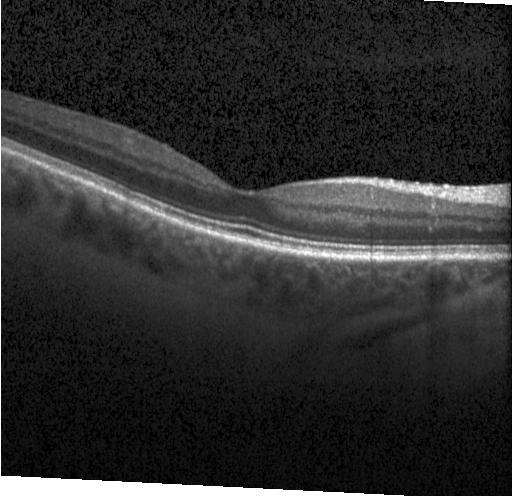

Impression: no choroidal neovascularization, no diabetic macular edema, and no drusen.